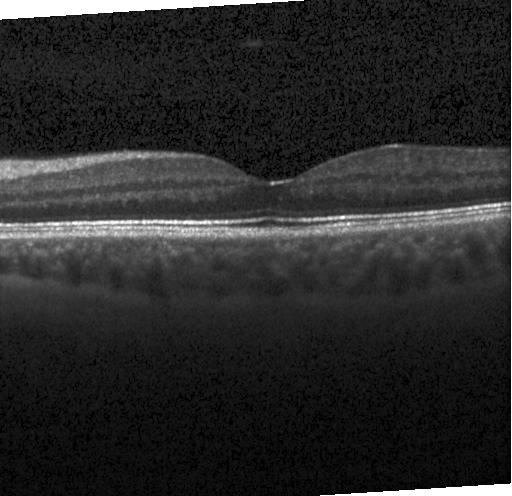 Optical coherence tomography scan — Assessment: neither choroidal neovascularization, diabetic macular edema, nor drusen.